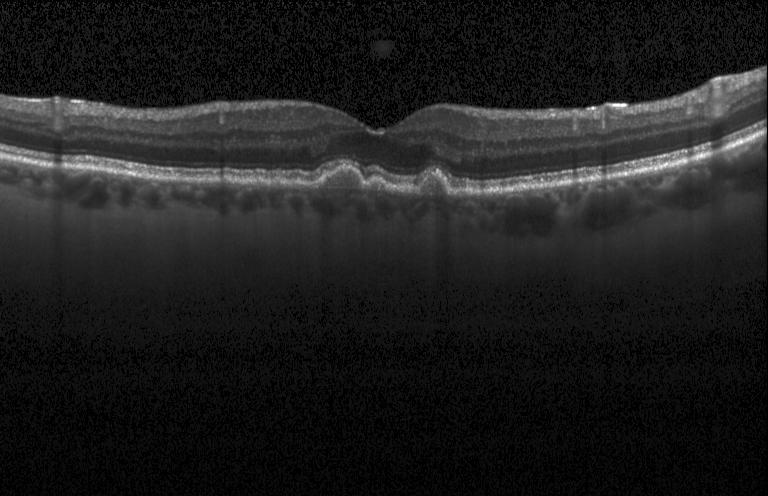 OCT scan showing drusen.